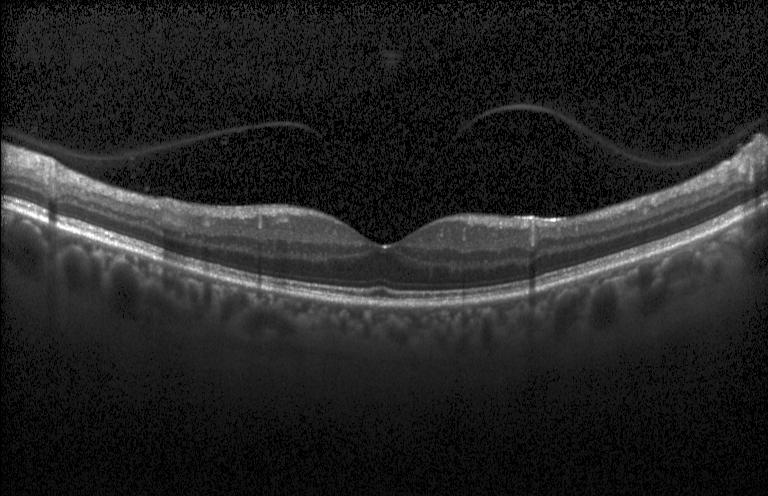

Through the macula; acquired on a Heidelberg Spectralis; OCT line scan. Assessment: no CNV, no DME, and no drusen.